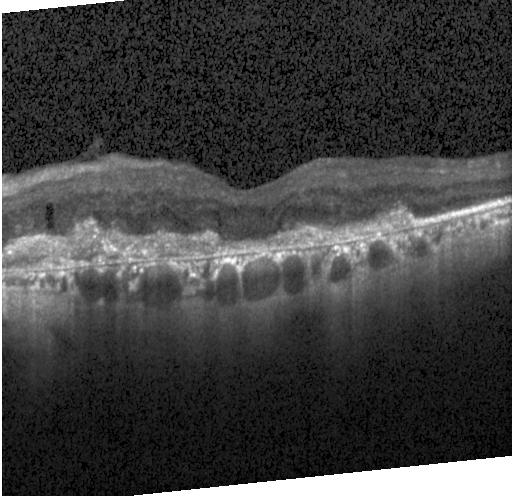

Finding: a choroidal neovascular membrane.